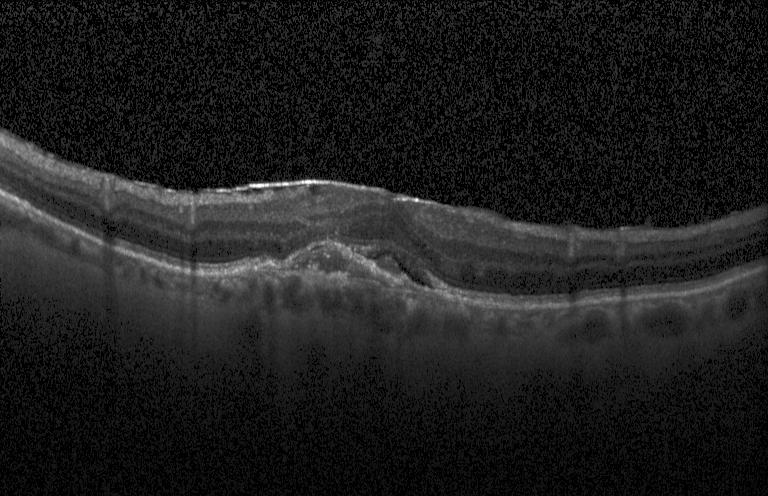

Retinal OCT cross-section — Impression: a choroidal neovascular membrane.